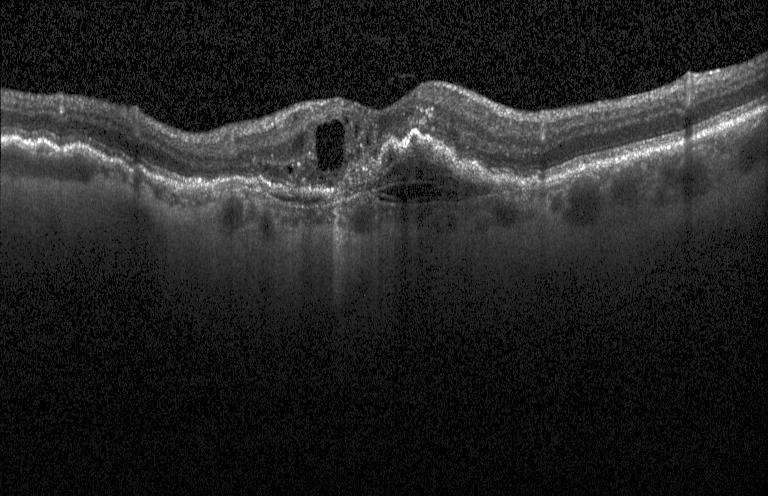
Retinal OCT cross-section · instrument: Heidelberg Spectralis
Finding: a choroidal neovascular membrane.